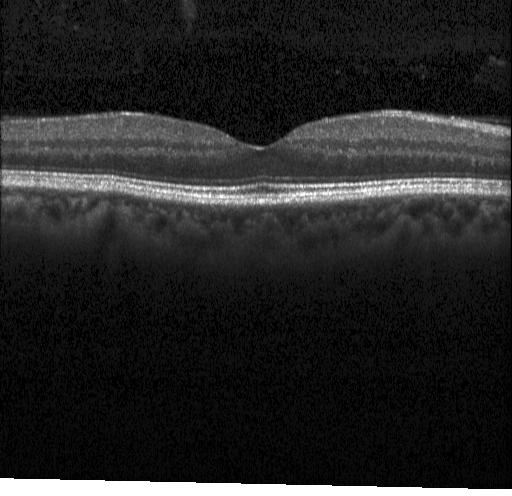 Heidelberg Spectralis; OCT B-scan — Impression: no choroidal neovascularization, no diabetic macular edema, and no drusen.